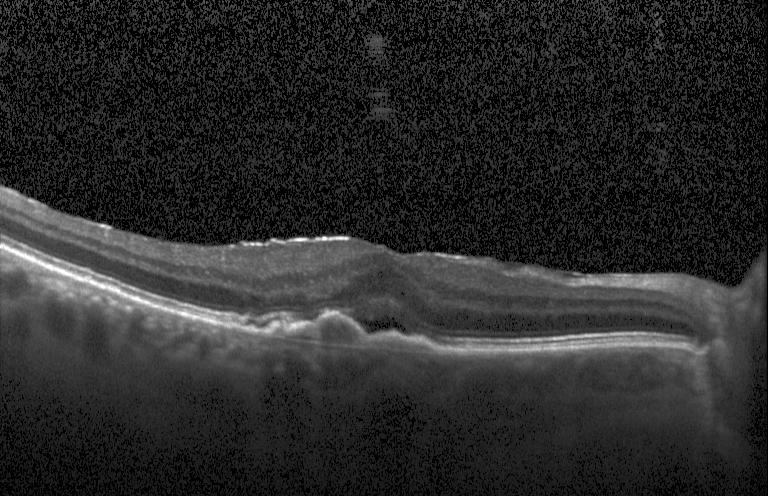

Retinal OCT cross-section showing choroidal neovascularization.